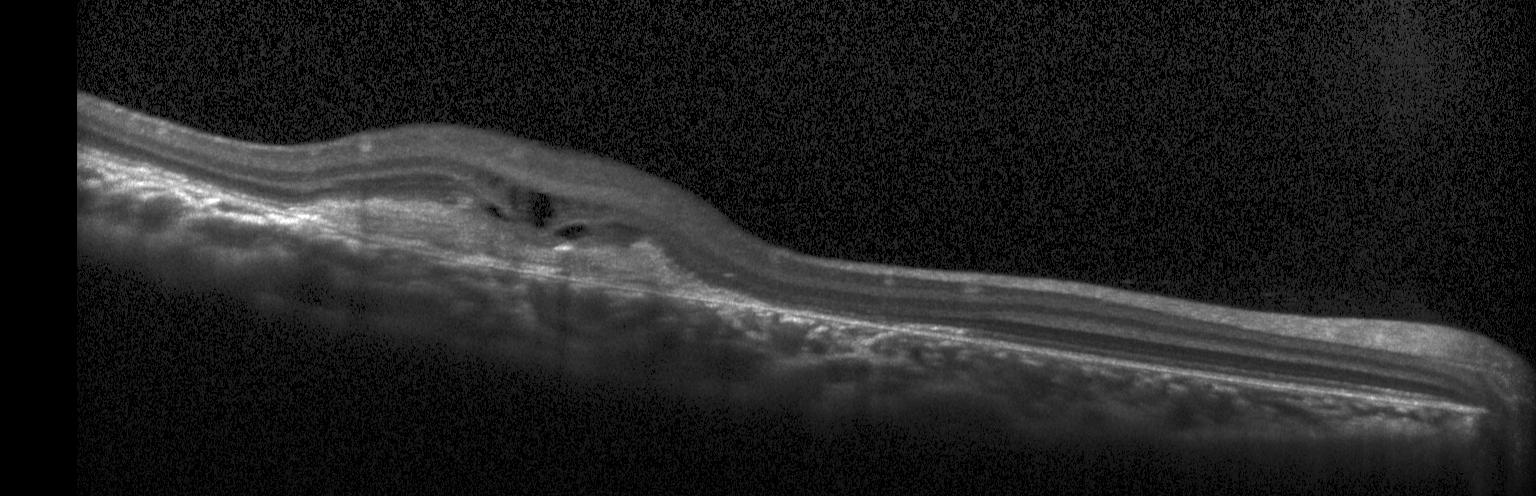

Optical coherence tomography B-scan, acquired on a Heidelberg Spectralis
Assessment: choroidal neovascularization.